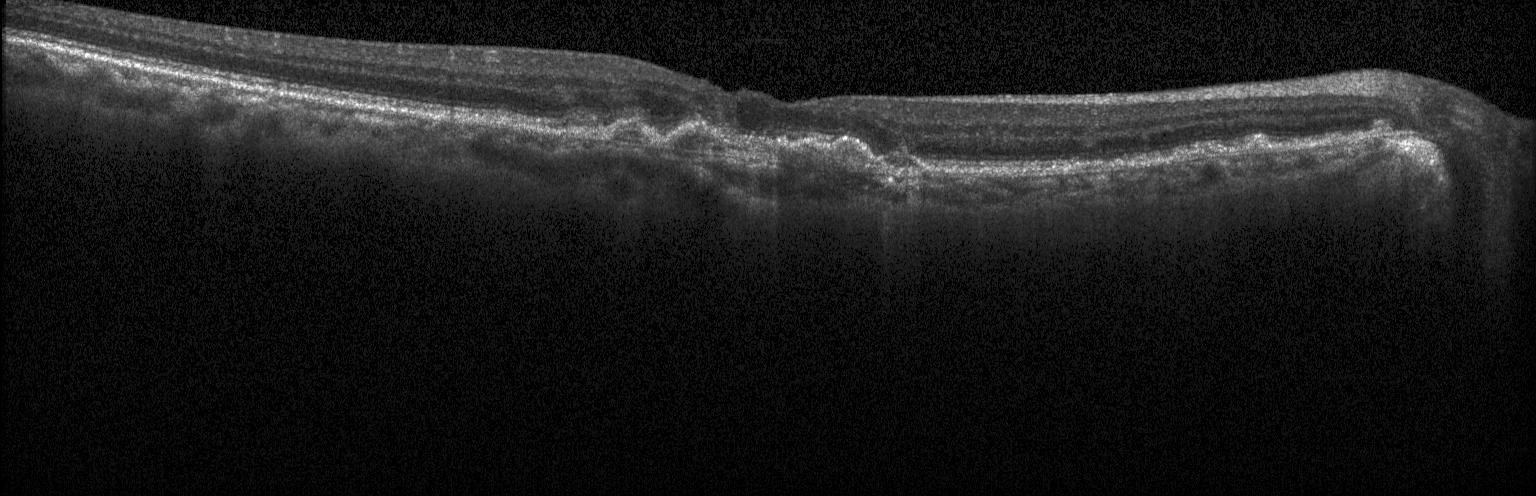

Diagnosis: a choroidal neovascular membrane.